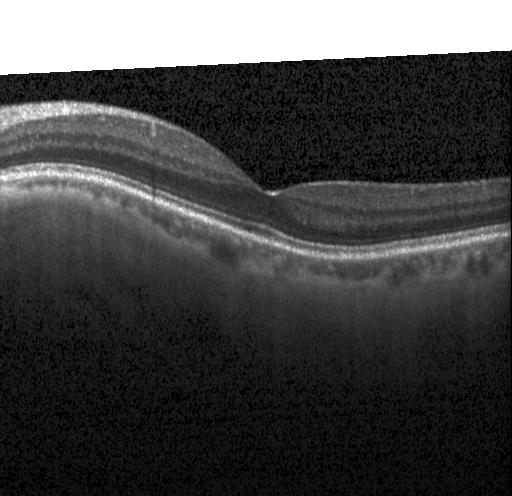 Instrument: Heidelberg Spectralis · optical coherence tomography scan — Dx: neither choroidal neovascularization, diabetic macular edema, nor drusen.